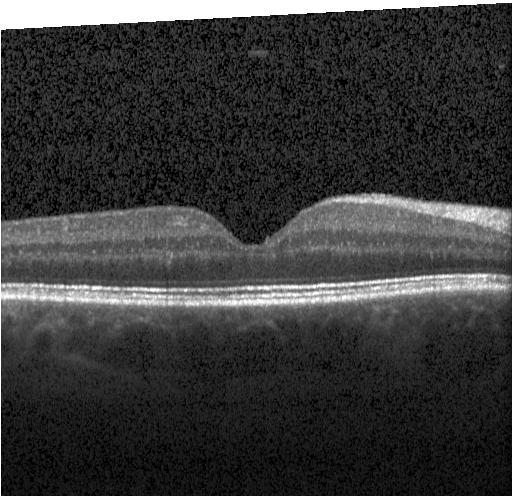

Spectral-domain OCT, macular scan, retinal OCT cross-section, acquired on a Heidelberg Spectralis — Finding: neither choroidal neovascularization, diabetic macular edema, nor drusen.